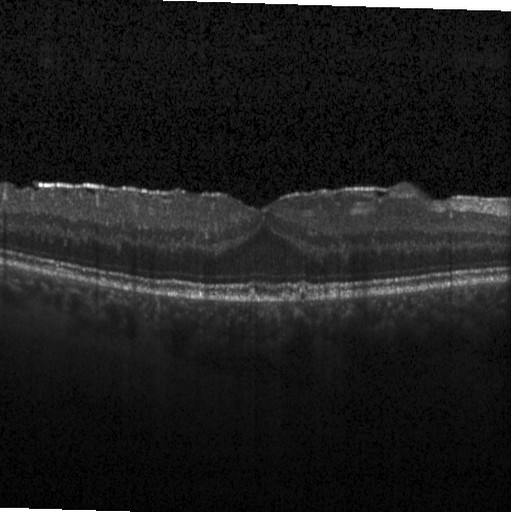 Diagnosis: diabetic macular edema (DME).